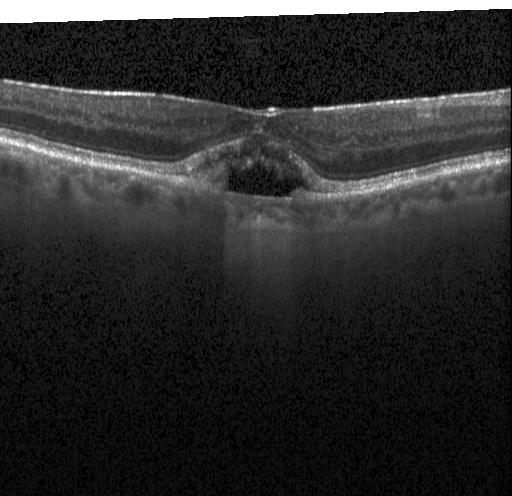 Retinal OCT cross-section showing a choroidal neovascular membrane.